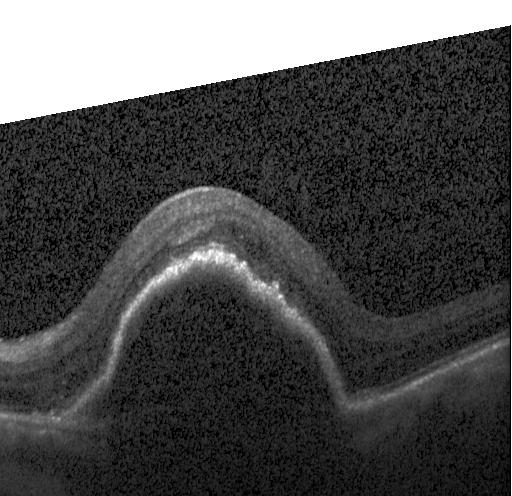 Macular OCT: a choroidal neovascular membrane.